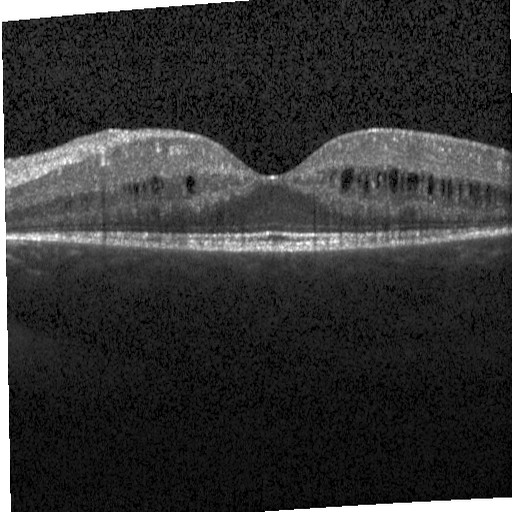

Spectral-domain OCT. Macular scan. Heidelberg Spectralis OCT system. Optical coherence tomography B-scan. Diabetic macular edema (DME).